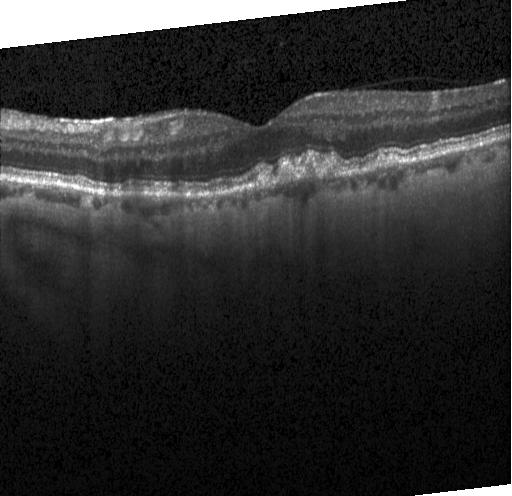 Optical coherence tomography B-scan · instrument: Heidelberg Spectralis. Macular OCT: drusen.